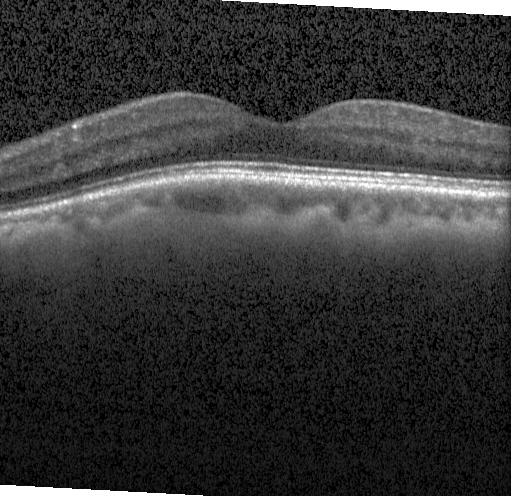 Instrument: Heidelberg Spectralis, through the macula, OCT line scan, spectral-domain optical coherence tomography.
Diagnosis: no CNV, DME, or drusen.